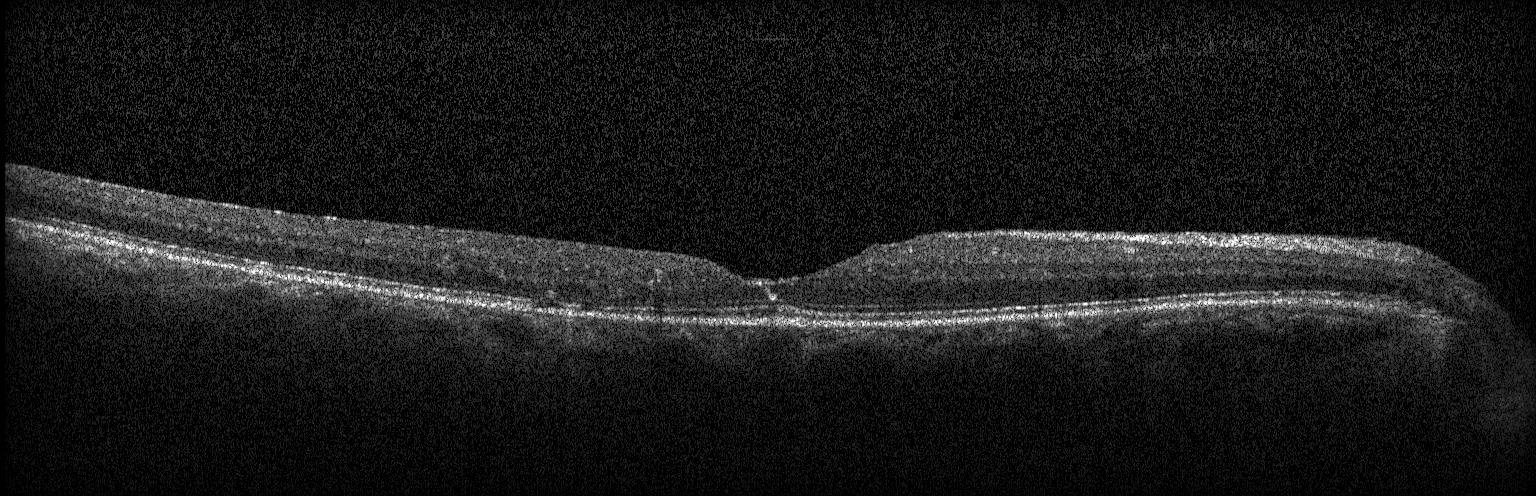 Optical coherence tomography B-scan — Diagnosis: no CNV, no DME, and no drusen.